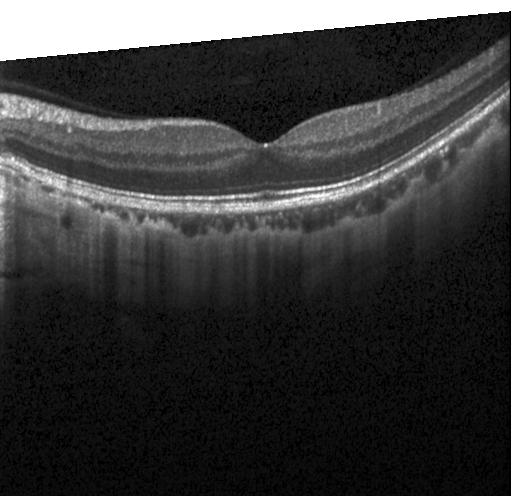
Impression: no choroidal neovascularization, no diabetic macular edema, and no drusen.